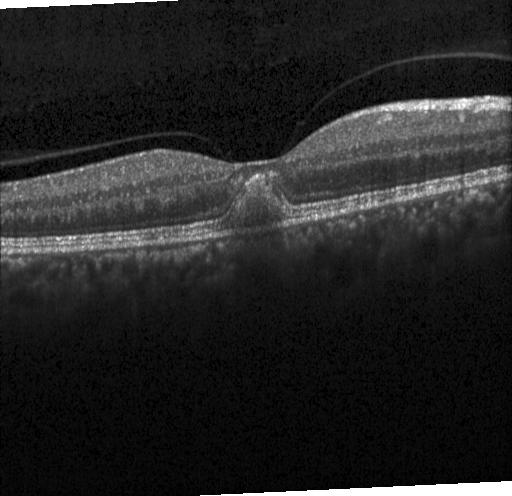 SD-OCT; OCT B-scan; horizontal scan through the fovea — The scan shows CNV.